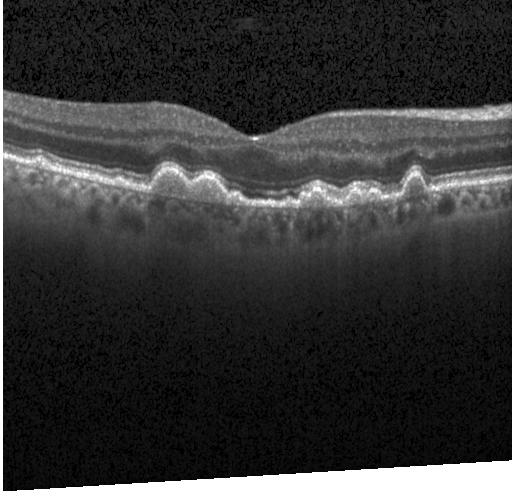

Optical coherence tomography B-scan.
Diagnosis: multiple drusen.